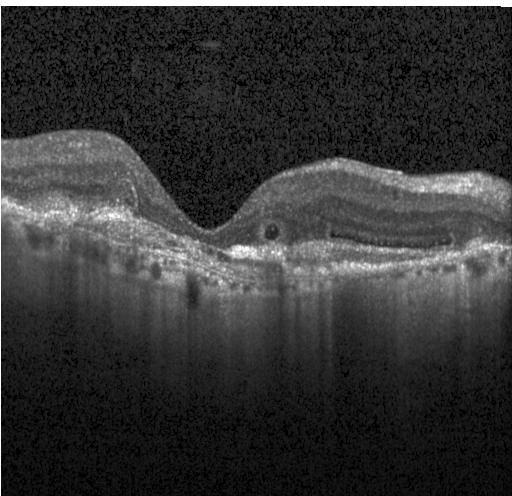

Diagnosis: choroidal neovascularization (CNV).